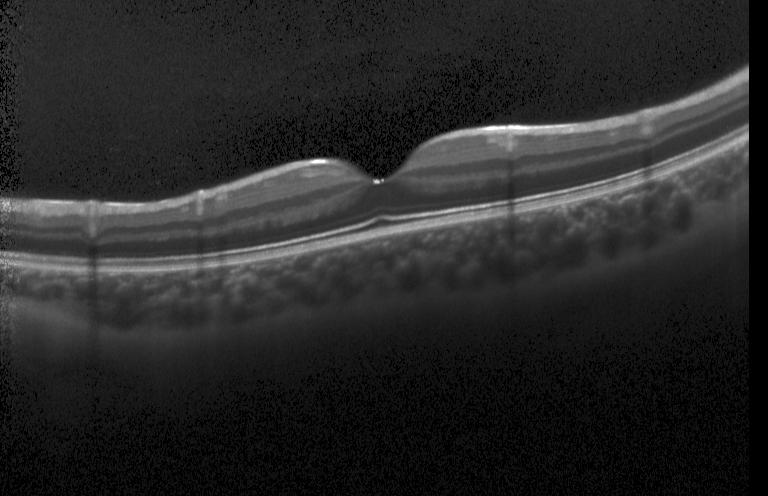

Retinal OCT cross-section · spectral-domain optical coherence tomography · Heidelberg Spectralis
Finding: neither choroidal neovascularization, diabetic macular edema, nor drusen.